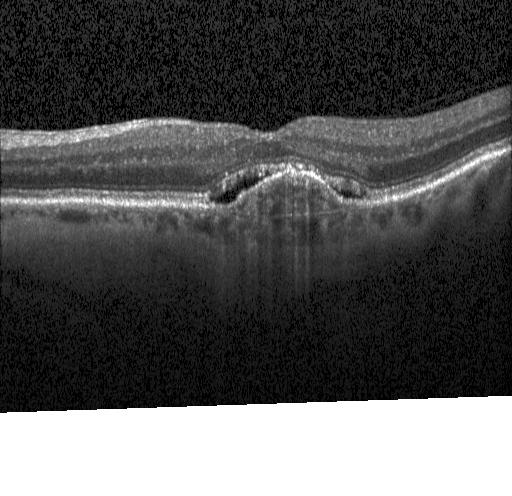
Heidelberg Spectralis OCT system; spectral-domain OCT; retinal OCT cross-section.
Diagnosis: a choroidal neovascular membrane.